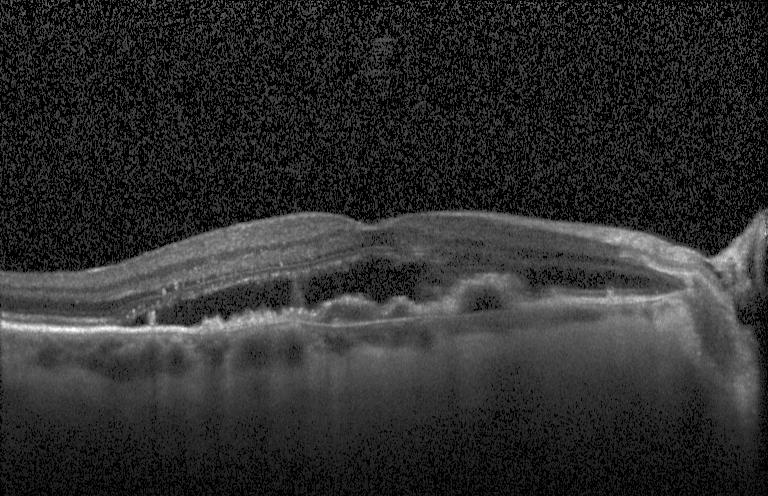

OCT B-scan, instrument: Heidelberg Spectralis
OCT finding: CNV.